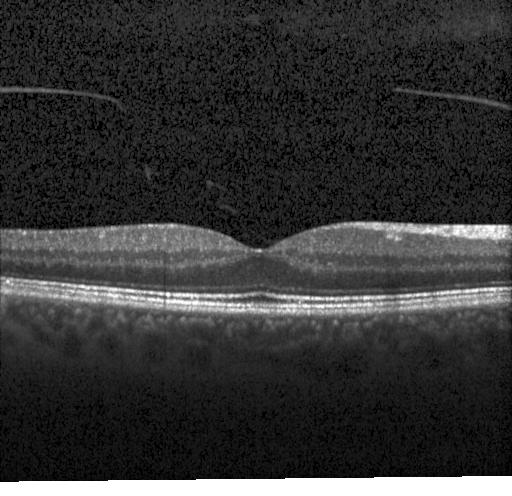

SD-OCT. Retinal OCT B-scan. Macular scan — Finding: no choroidal neovascularization, no diabetic macular edema, and no drusen.